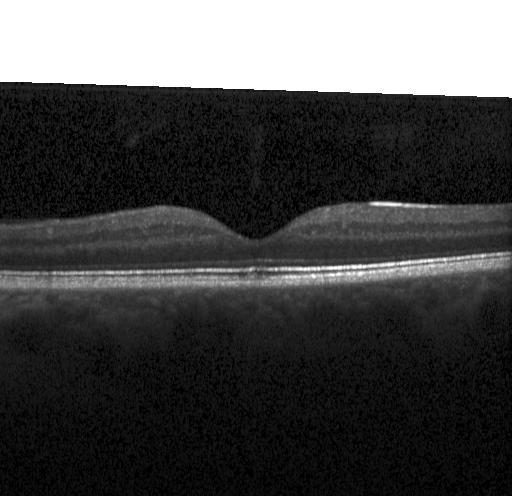

OCT B-scan showing no evidence of choroidal neovascularization, diabetic macular edema, or drusen.